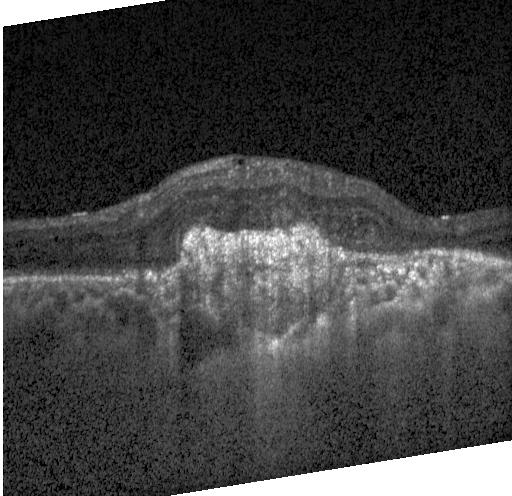

Optical coherence tomography scan — Impression: choroidal neovascularization (CNV).